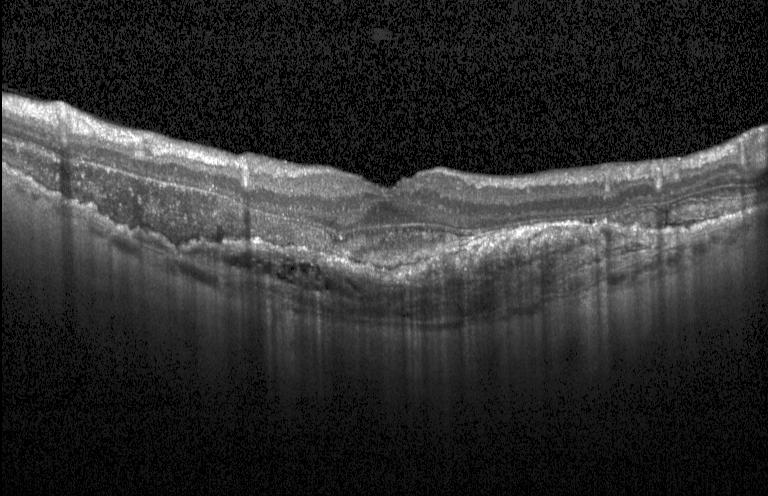
Macular scan, acquired on a Heidelberg Spectralis, optical coherence tomography B-scan
Macular OCT: a choroidal neovascular membrane.